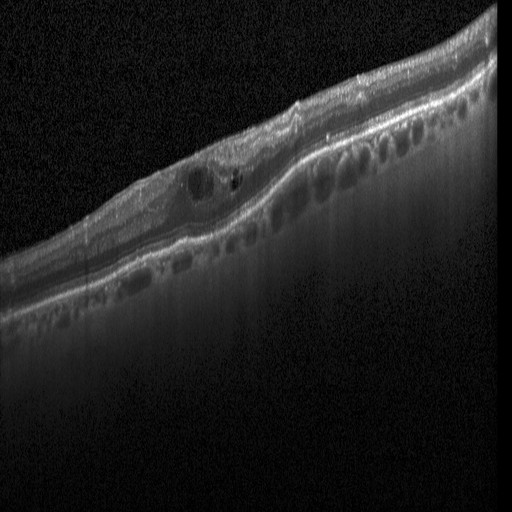

SD-OCT. Retinal OCT cross-section
Dx: diabetic macular edema.